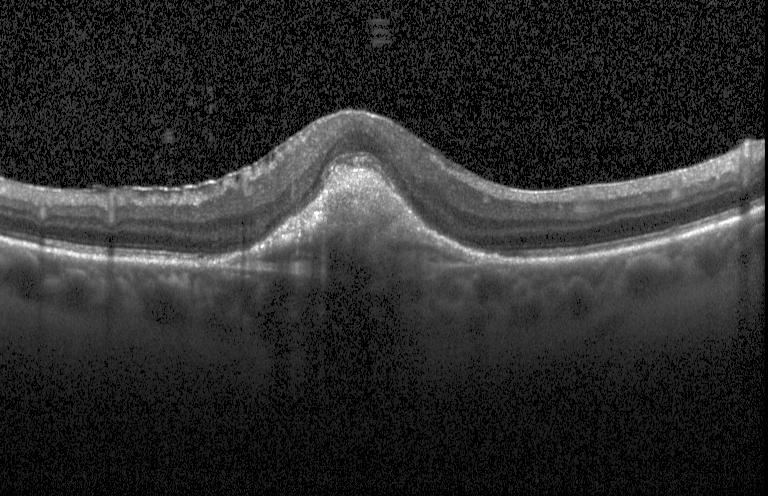 OCT B-scan showing choroidal neovascularization (CNV).